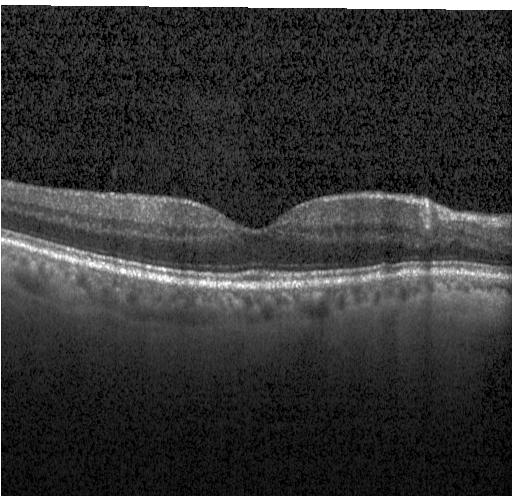 OCT line scan, fovea-centered
Impression: neither CNV, DME, nor drusen.